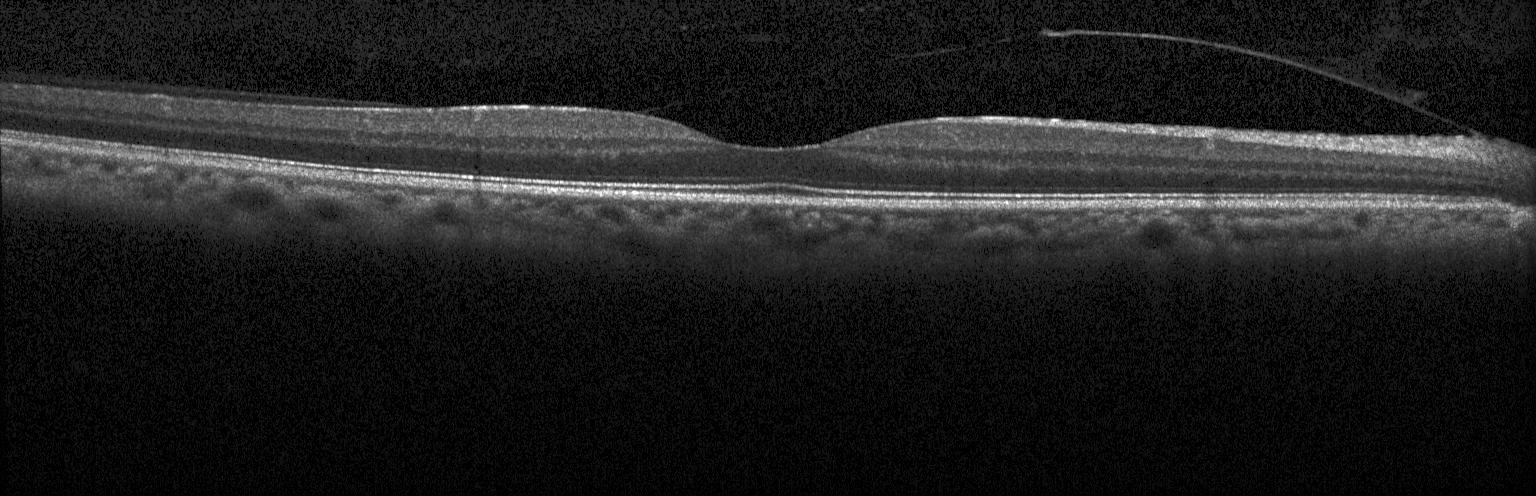
Neither choroidal neovascularization, diabetic macular edema, nor drusen.